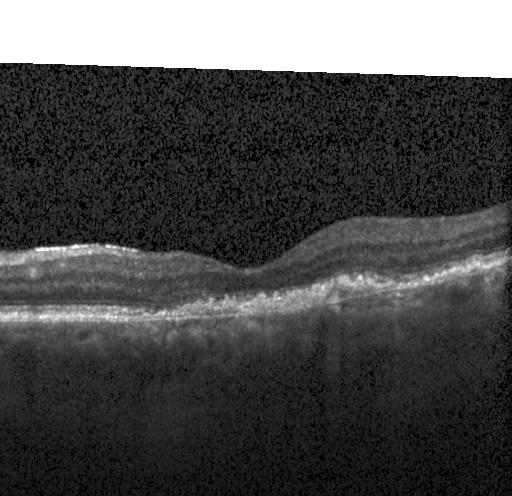 Through the macula. Instrument: Heidelberg Spectralis. Retinal OCT B-scan. SD-OCT — The scan shows choroidal neovascularization (CNV).